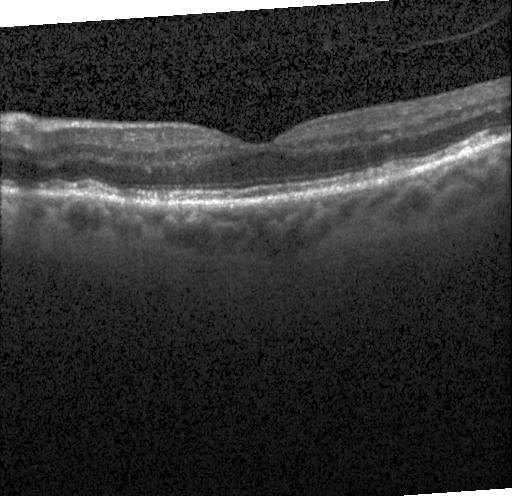 OCT B-scan
Diagnosis: sub-RPE drusenoid deposits.